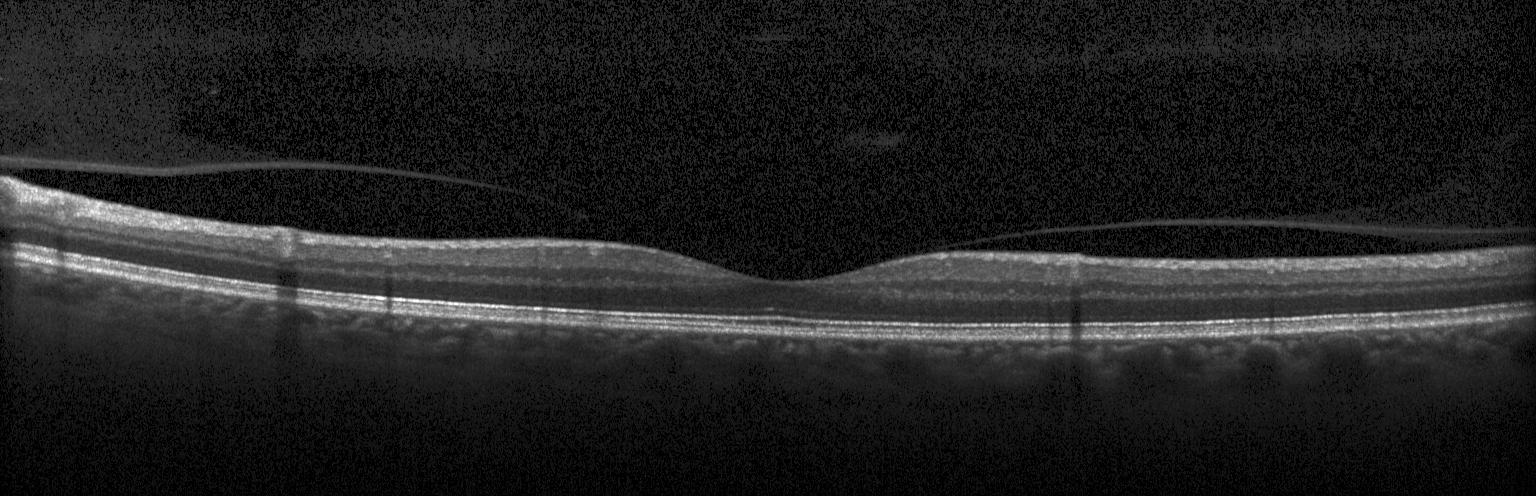

Spectral-domain optical coherence tomography; retinal OCT B-scan; centered on the fovea. Finding: no CNV, DME, or drusen.